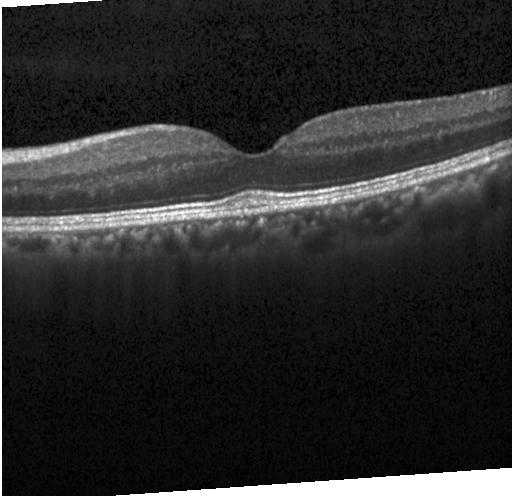
Neither choroidal neovascularization, diabetic macular edema, nor drusen.